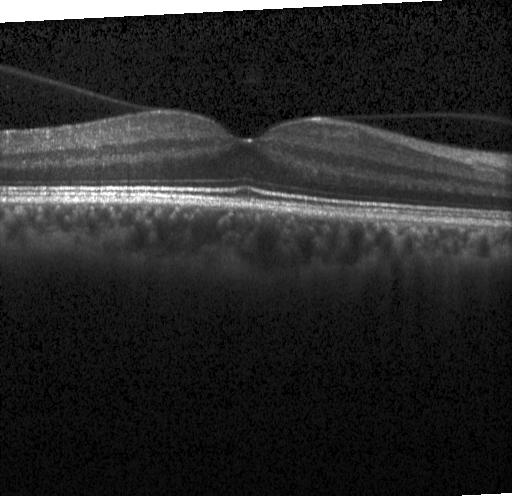 OCT B-scan. SD-OCT
The scan shows neither choroidal neovascularization, diabetic macular edema, nor drusen.